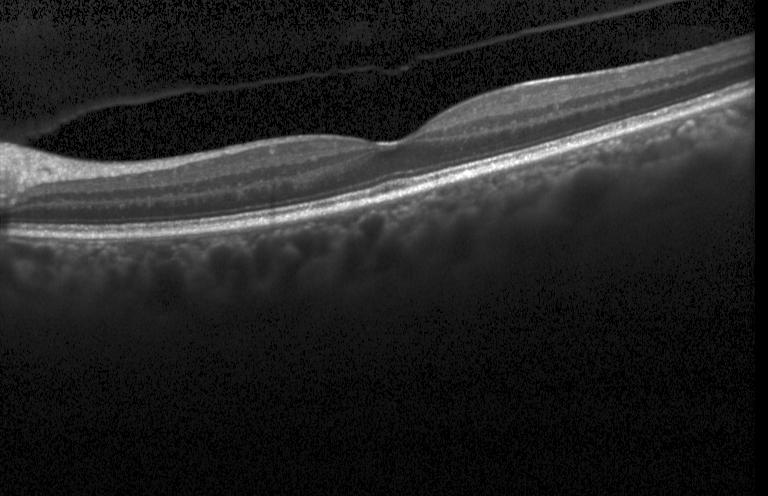 Optical coherence tomography scan; spectral-domain optical coherence tomography — Finding: neither CNV, DME, nor drusen.